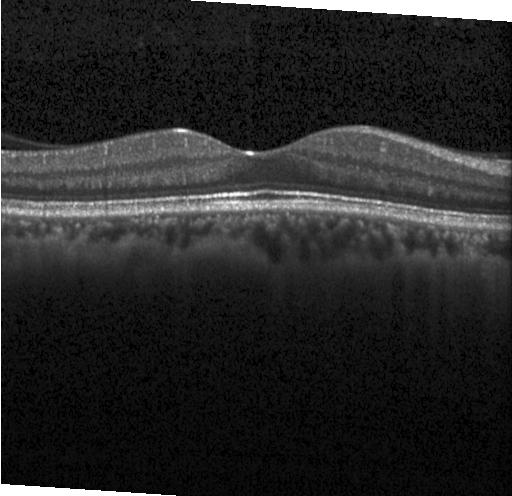 Instrument: Heidelberg Spectralis; SD-OCT; OCT line scan; fovea-centered. Dx: no CNV, DME, or drusen.